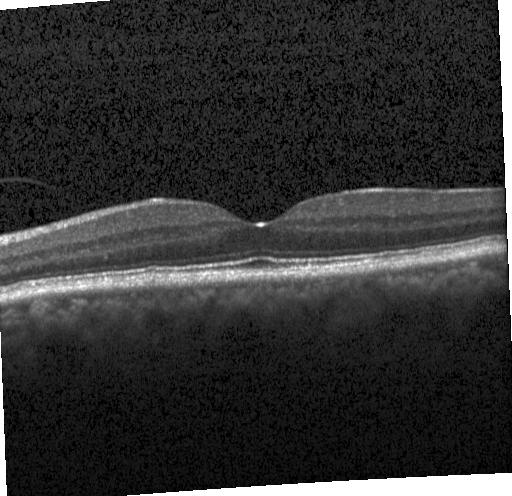 Finding: no CNV, no DME, and no drusen.